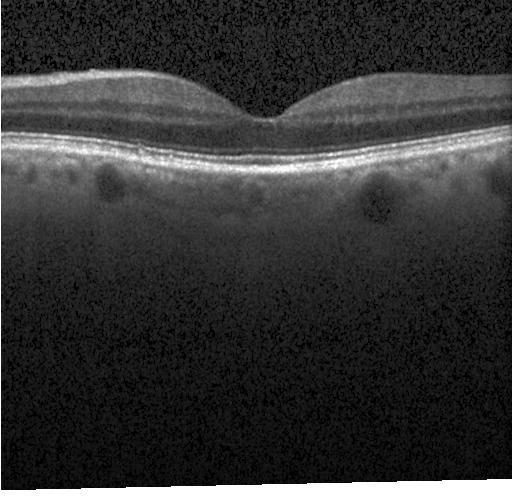 Diagnosis: no evidence of CNV, DME, or drusen.